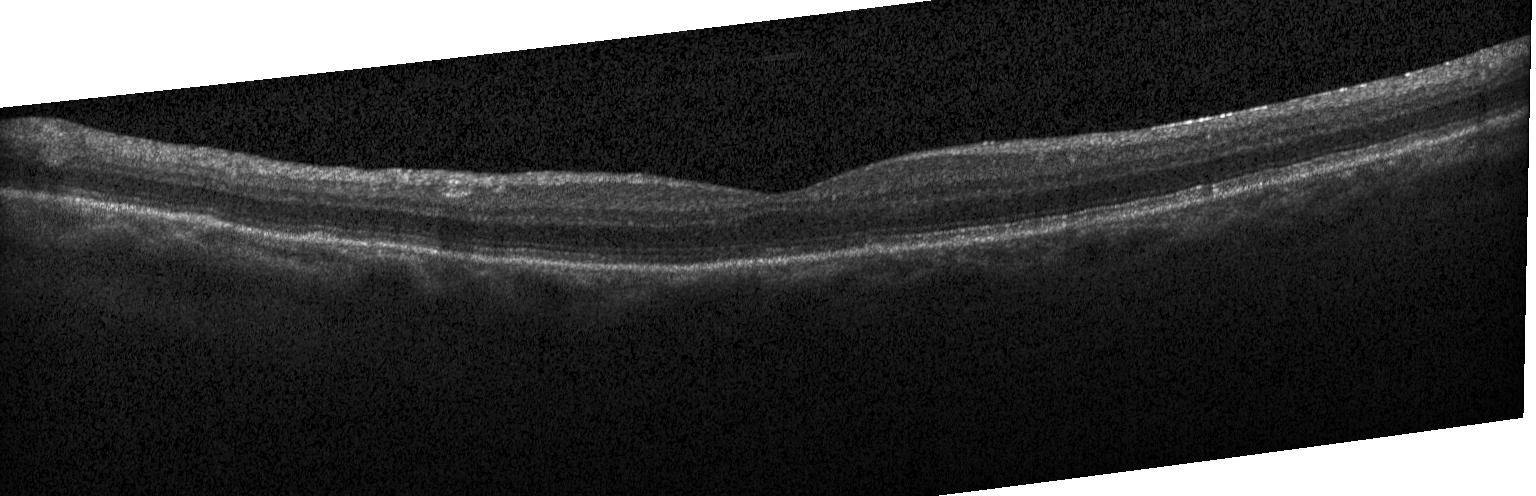

Impression: sub-RPE drusenoid deposits.